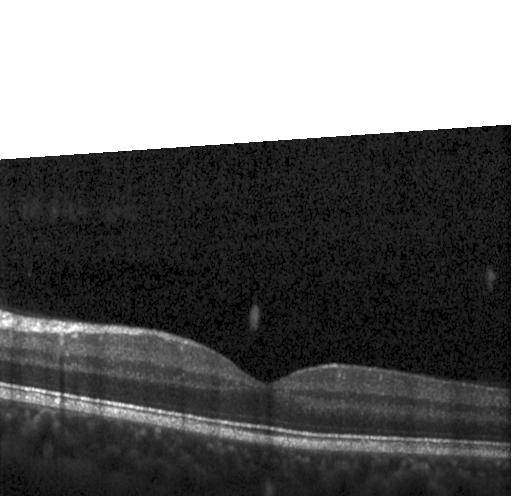

Optical coherence tomography scan — The scan shows no CNV, DME, or drusen.